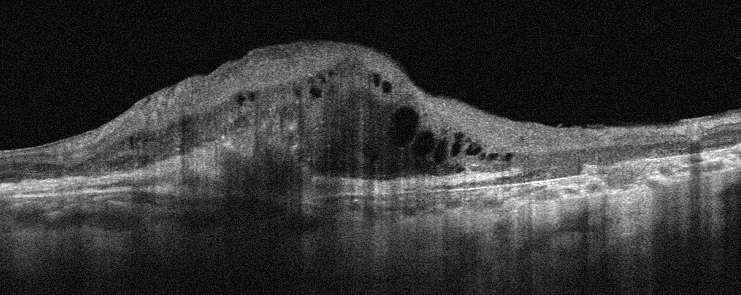

OCT line scan; fovea-centered.
Finding: age-related macular degeneration (AMD).